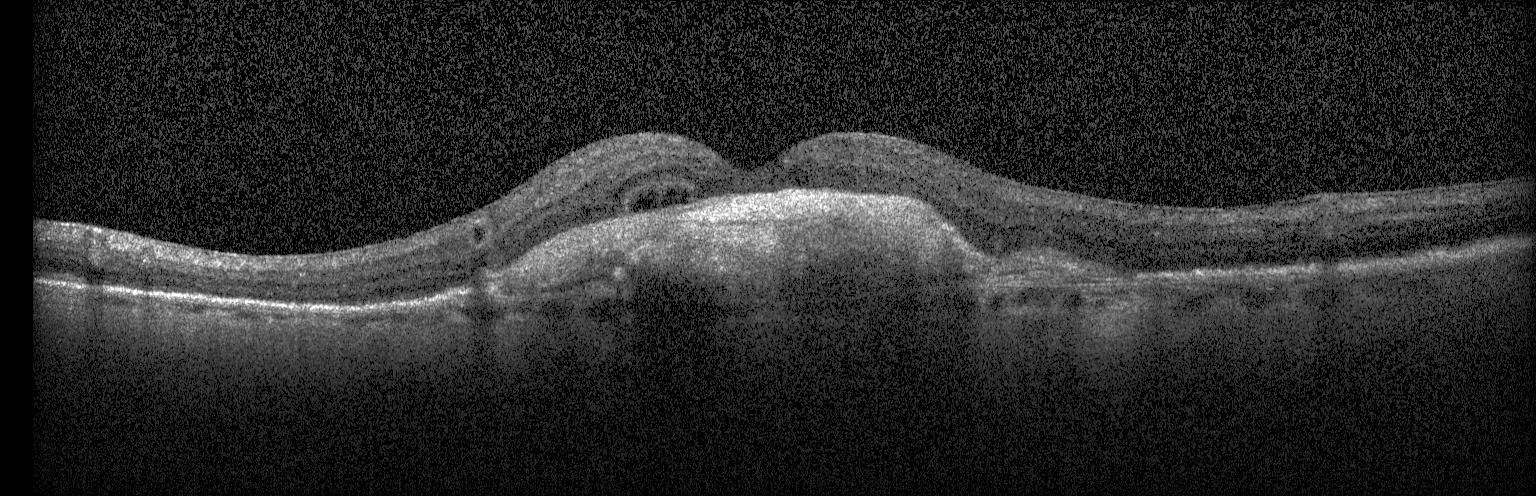 Retinal OCT cross-section. A choroidal neovascular membrane.